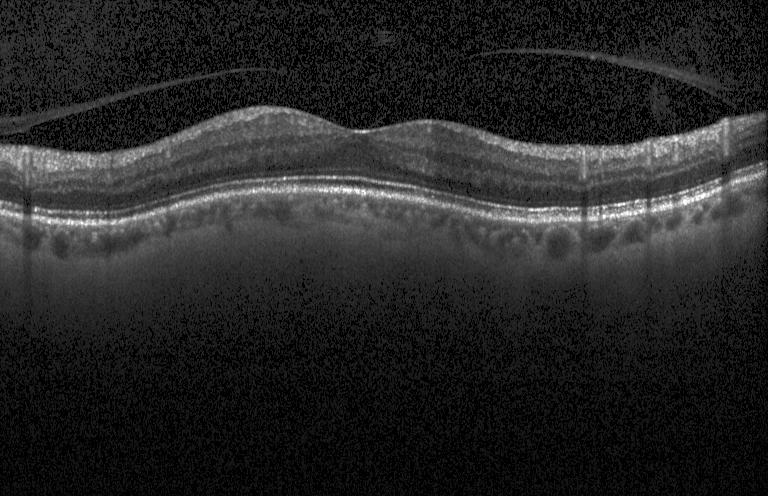 Optical coherence tomography B-scan. This B-scan demonstrates no choroidal neovascularization, no diabetic macular edema, and no drusen.